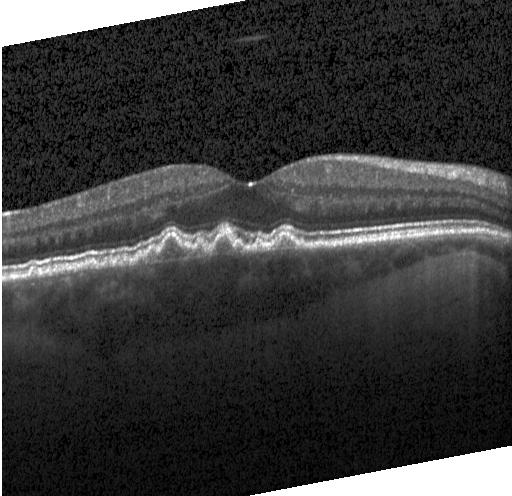 Heidelberg Spectralis; optical coherence tomography scan. Multiple drusen.